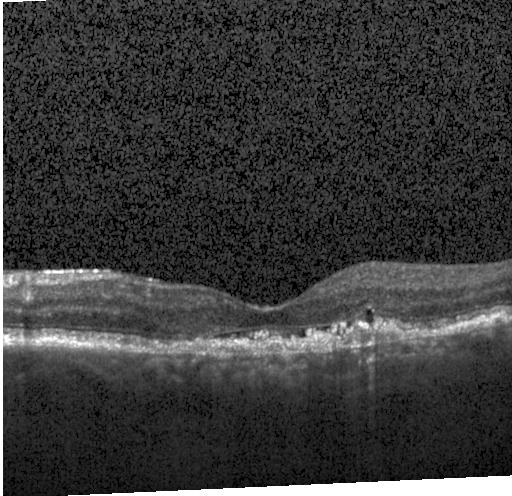 Fovea-centered · Heidelberg Spectralis OCT system · optical coherence tomography scan — Finding: a choroidal neovascular membrane.